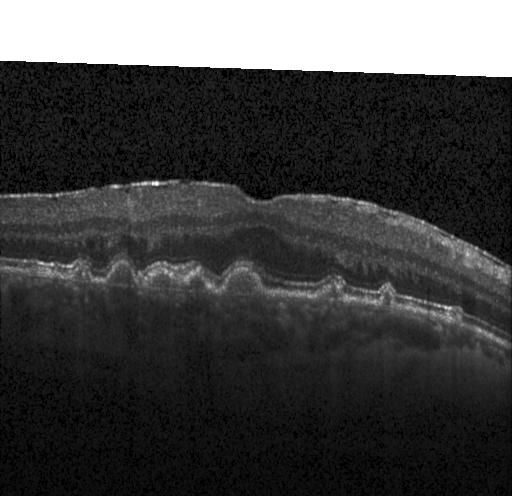

Spectral-domain OCT B-scan: multiple drusen.